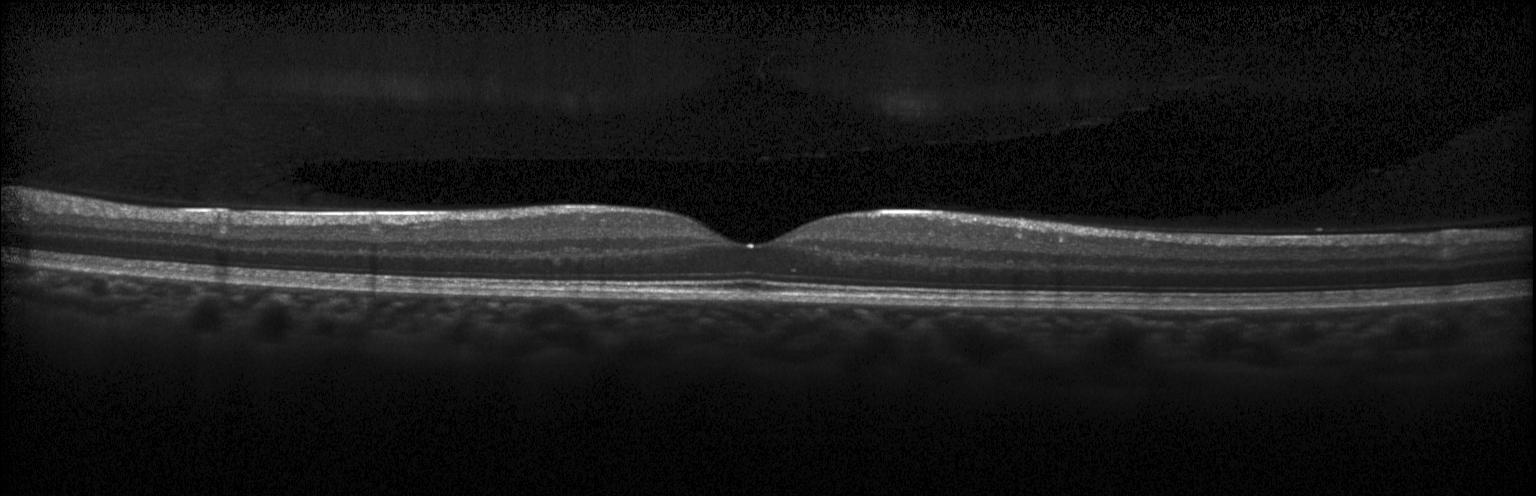 Finding: no evidence of CNV, DME, or drusen.